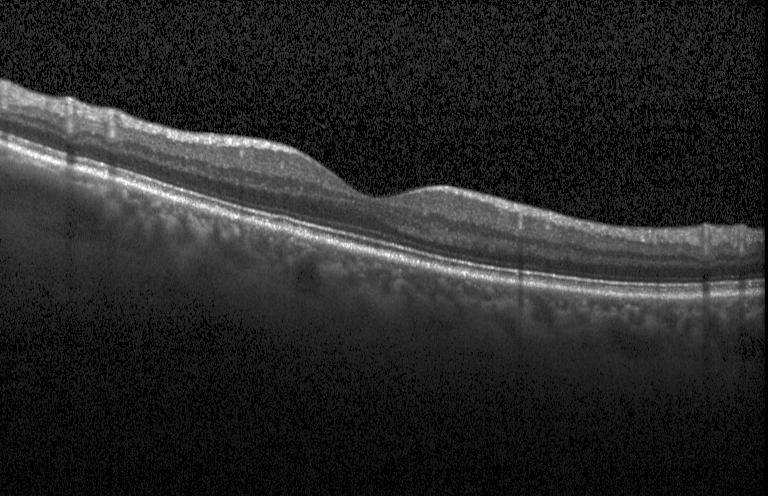

Instrument: Heidelberg Spectralis. Optical coherence tomography B-scan — Finding: no CNV, no DME, and no drusen.